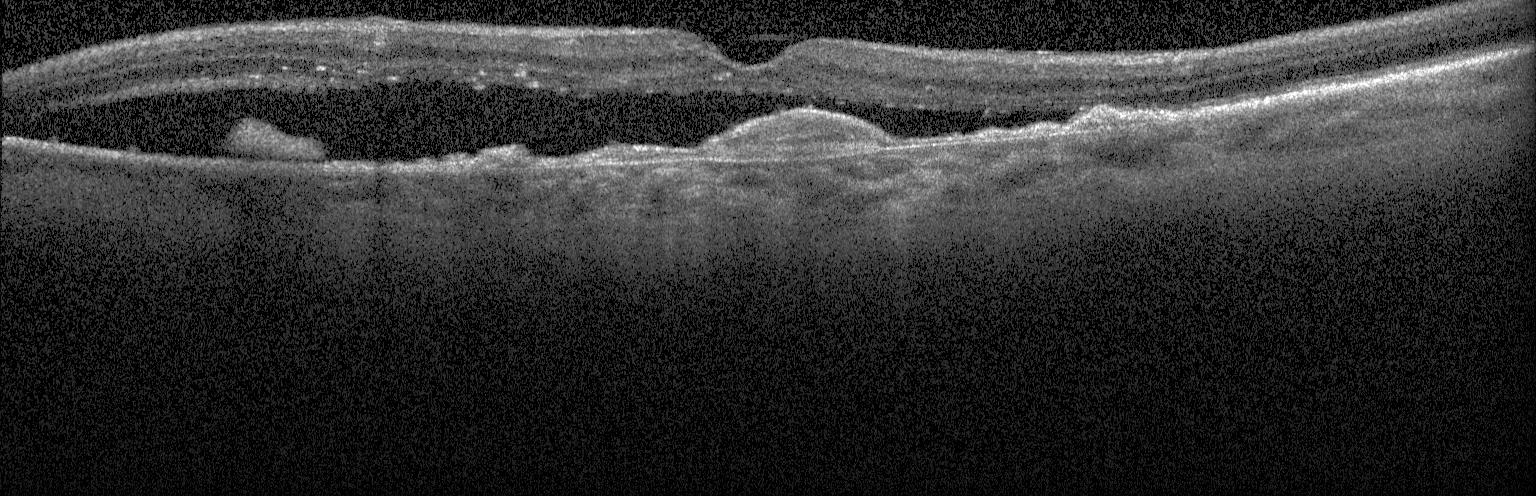 Retinal OCT cross-section · Heidelberg Spectralis OCT system · centered on the fovea · SD-OCT — Diagnosis: a choroidal neovascular membrane.